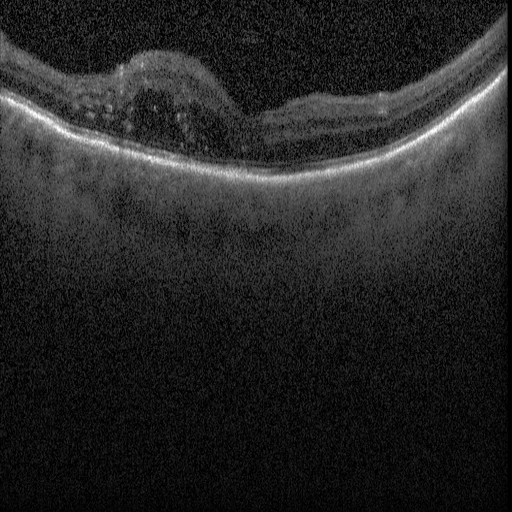

Acquired on a Heidelberg Spectralis, spectral-domain OCT, retinal OCT B-scan. This B-scan demonstrates DME.